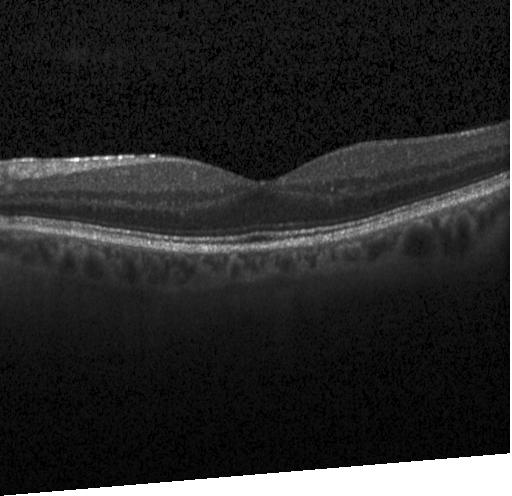

Instrument: Heidelberg Spectralis. Optical coherence tomography scan — Impression: no evidence of CNV, DME, or drusen.